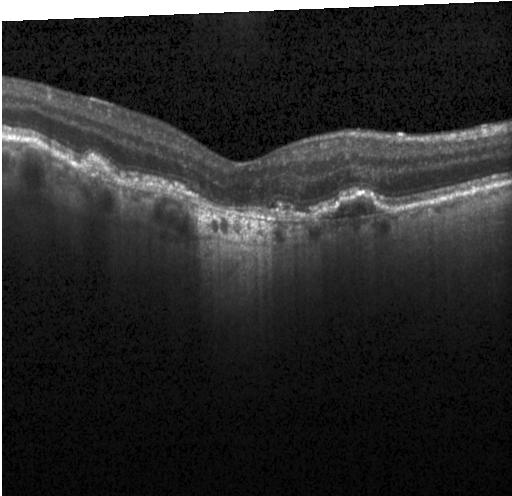
Instrument: Heidelberg Spectralis · optical coherence tomography B-scan · fovea-centered.
Impression: choroidal neovascularization.